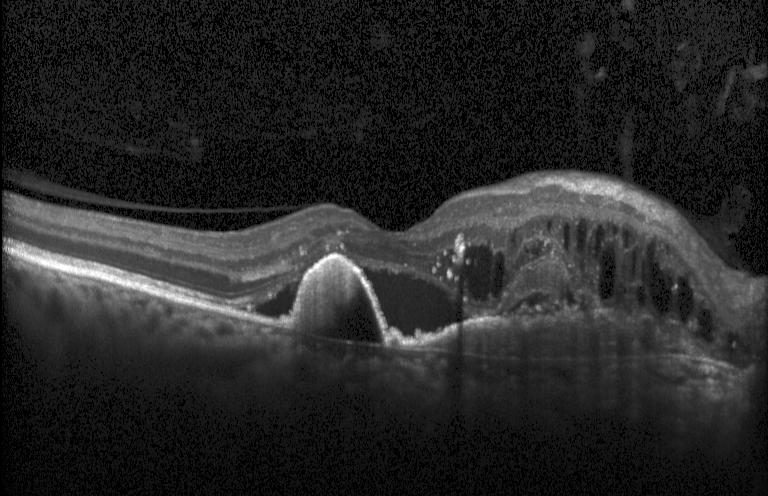

Optical coherence tomography B-scan. Spectral-domain optical coherence tomography. OCT finding: a choroidal neovascular membrane.